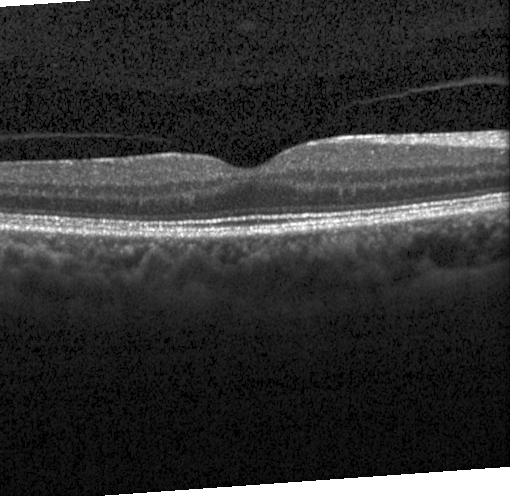
Instrument: Heidelberg Spectralis · OCT B-scan — Finding: neither choroidal neovascularization, diabetic macular edema, nor drusen.